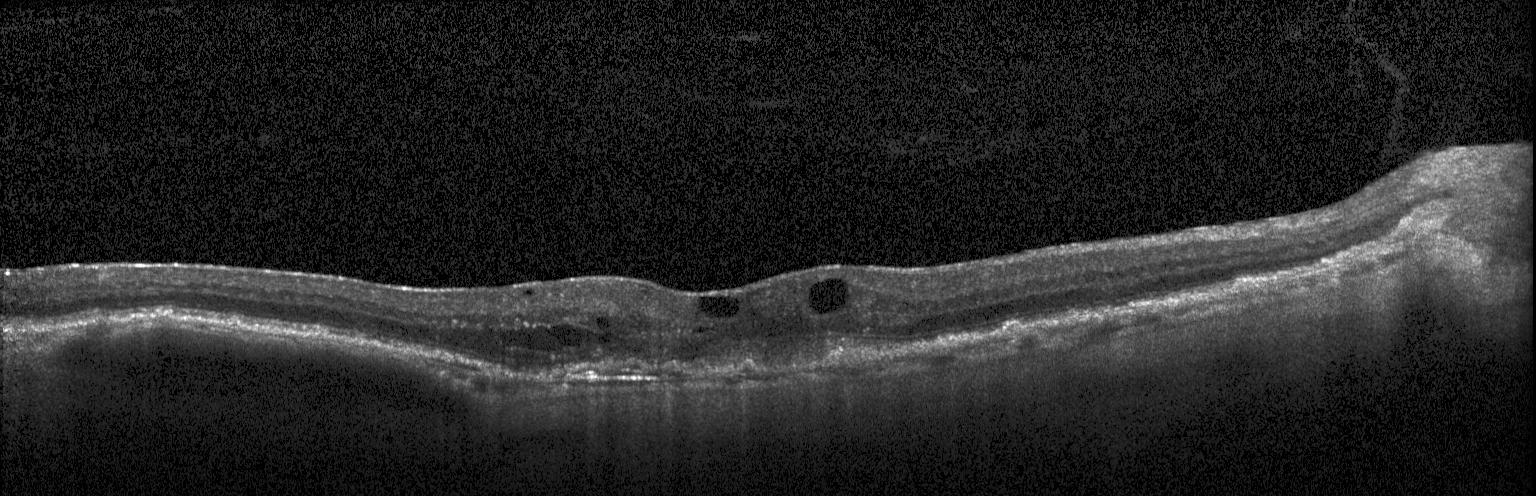

Finding: CNV.